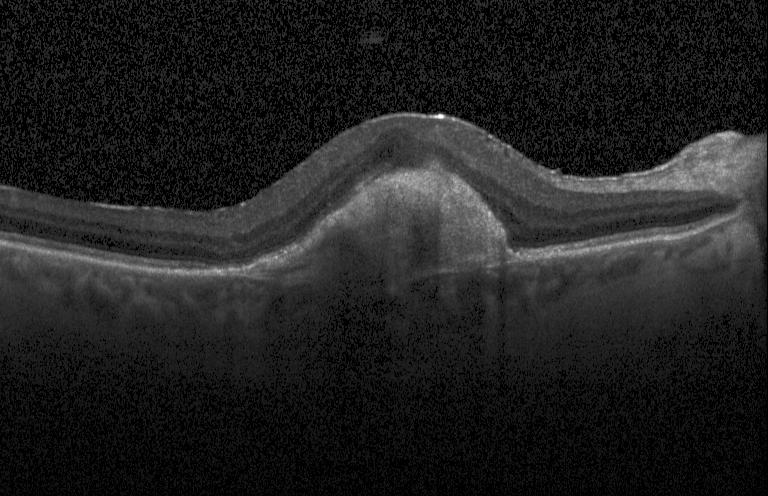 Macular OCT demonstrating a choroidal neovascular membrane.